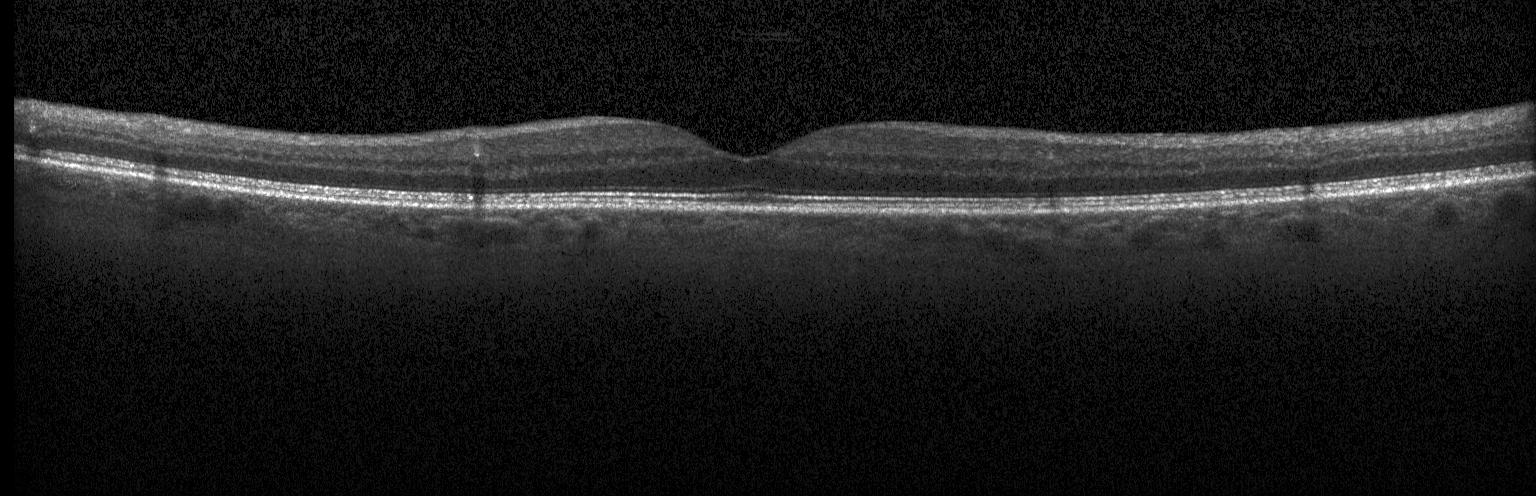
Macular OCT: no evidence of choroidal neovascularization, diabetic macular edema, or drusen.